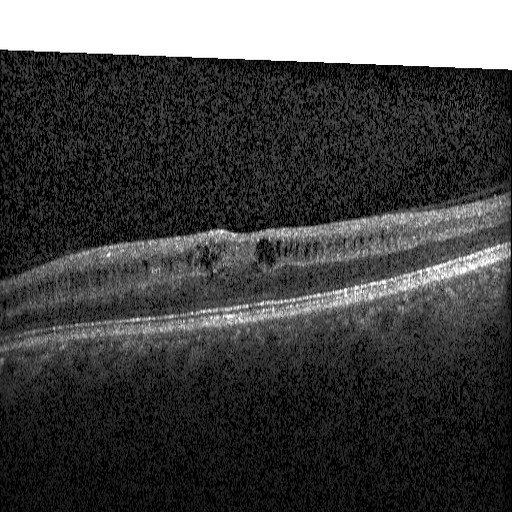

Optical coherence tomography scan.
Impression: diabetic macular edema (DME).